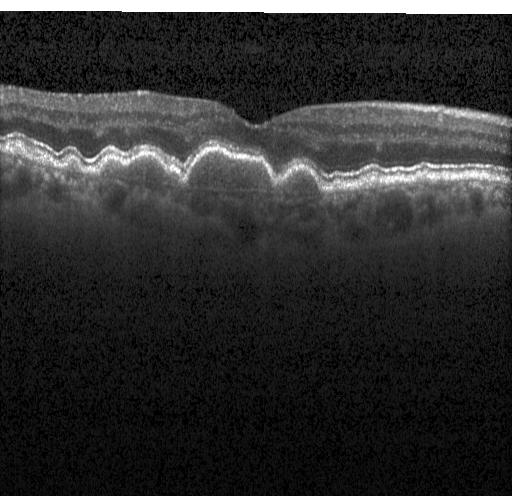 Retinal OCT cross-section showing sub-RPE drusenoid deposits.